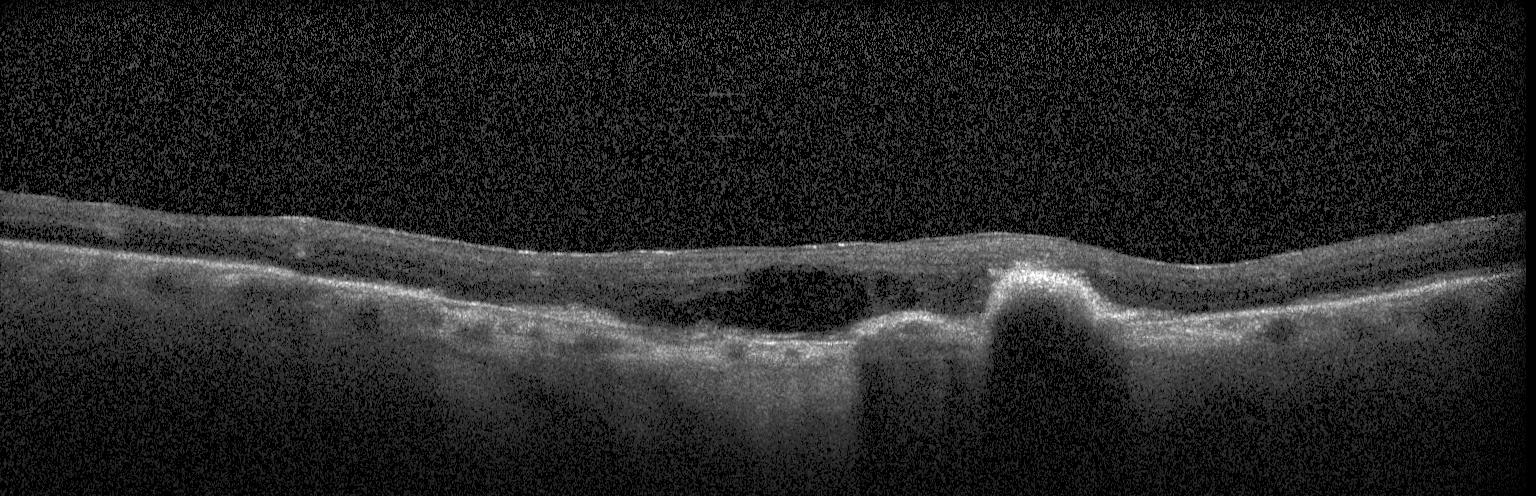 Optical coherence tomography B-scan.
OCT finding: a choroidal neovascular membrane.